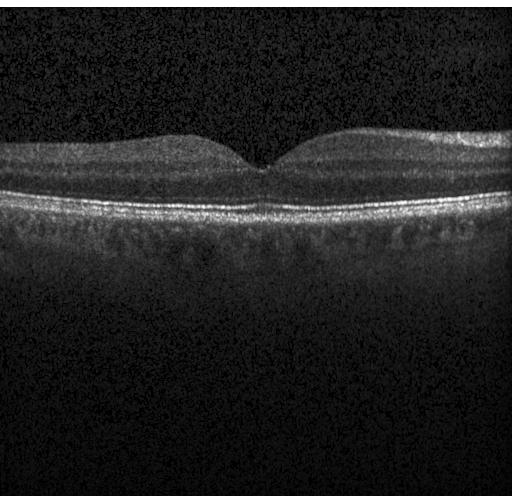

OCT B-scan showing neither choroidal neovascularization, diabetic macular edema, nor drusen.